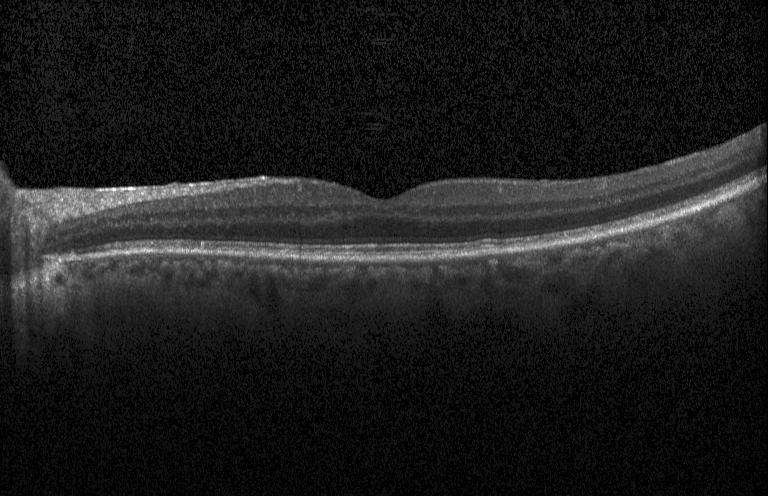 Finding: no choroidal neovascularization, no diabetic macular edema, and no drusen.